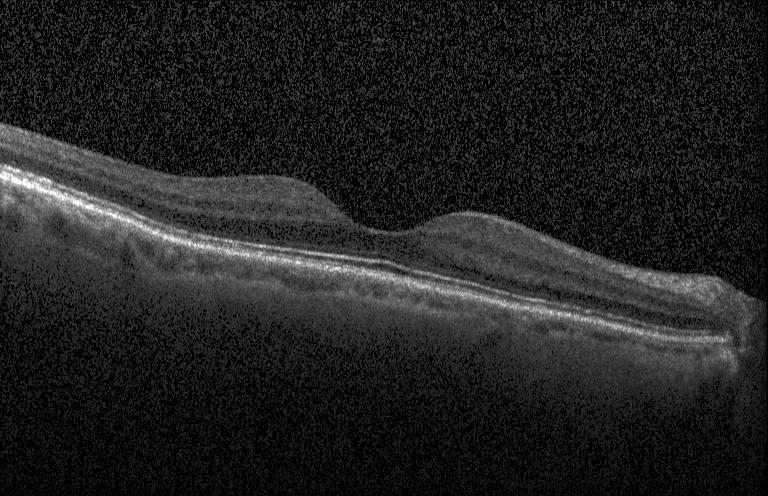
Retinal OCT cross-section. Heidelberg Spectralis. Horizontal scan through the fovea
Finding: neither choroidal neovascularization, diabetic macular edema, nor drusen.